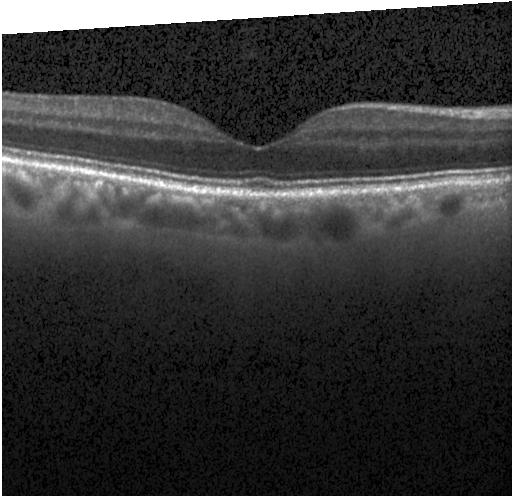

Centered on the fovea; spectral-domain OCT; OCT B-scan
Finding: no choroidal neovascularization, no diabetic macular edema, and no drusen.